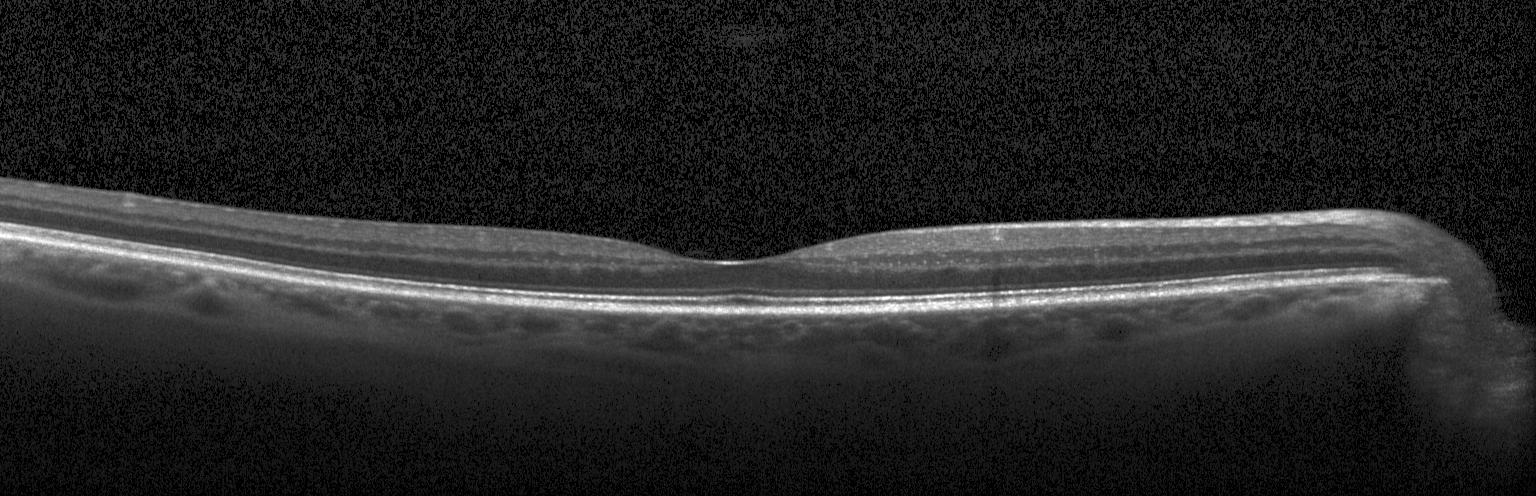 Macular OCT: neither choroidal neovascularization, diabetic macular edema, nor drusen.